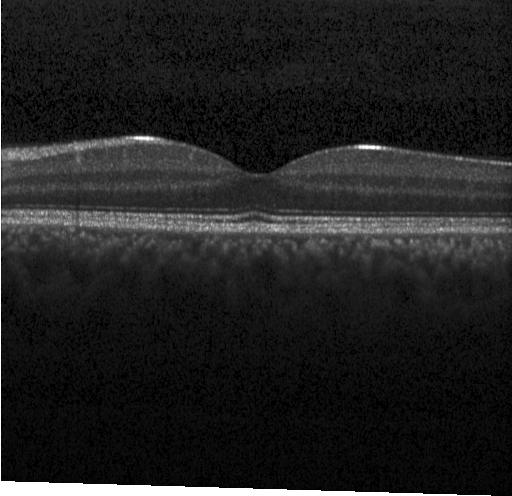
Spectral-domain OCT, instrument: Heidelberg Spectralis, centered on the fovea, retinal OCT cross-section. Finding: no choroidal neovascularization, diabetic macular edema, or drusen.